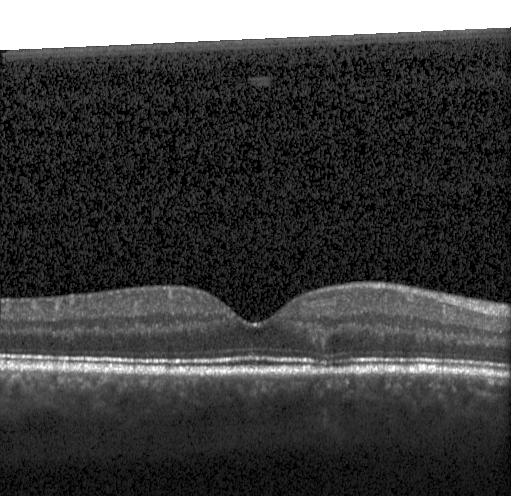 OCT line scan.
Macular OCT: neither CNV, DME, nor drusen.